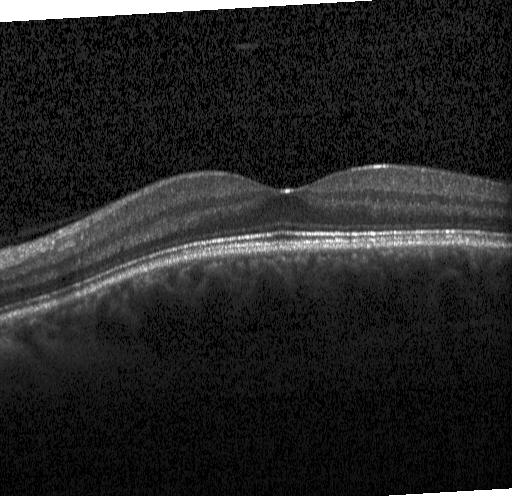 SD-OCT · OCT B-scan
This B-scan demonstrates neither choroidal neovascularization, diabetic macular edema, nor drusen.